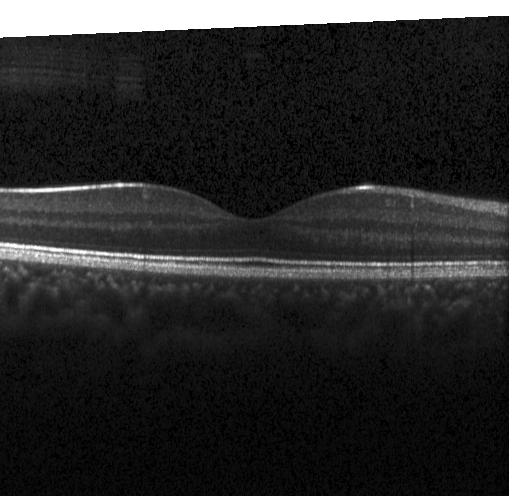
Centered on the fovea · optical coherence tomography B-scan · spectral-domain OCT · Heidelberg Spectralis
Finding: no evidence of choroidal neovascularization, diabetic macular edema, or drusen.